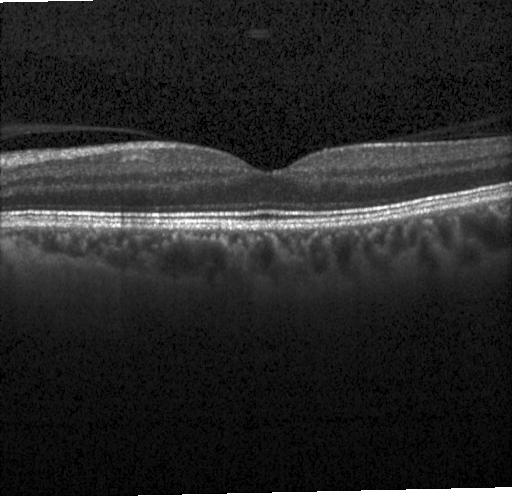 Centered on the fovea · acquired on a Heidelberg Spectralis · SD-OCT · optical coherence tomography B-scan — Macular OCT: no choroidal neovascularization, no diabetic macular edema, and no drusen.